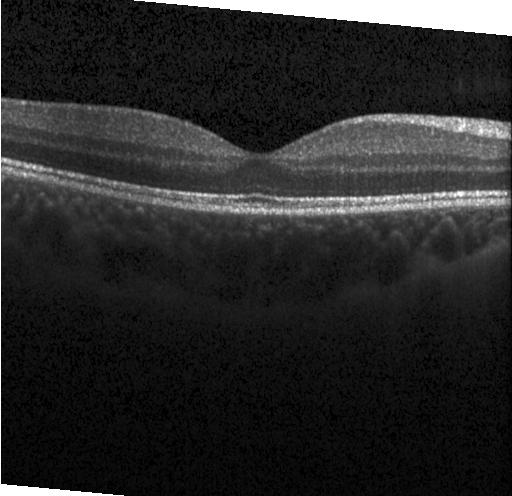
No choroidal neovascularization, no diabetic macular edema, and no drusen.